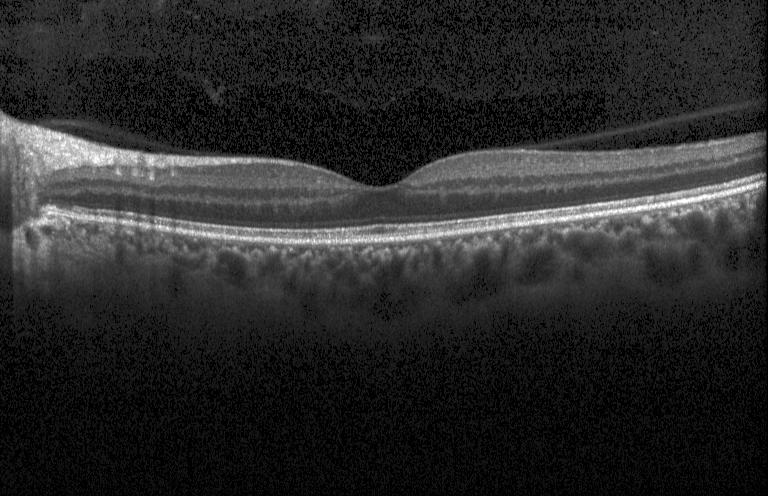
SD-OCT. OCT line scan
The scan shows no choroidal neovascularization, no diabetic macular edema, and no drusen.